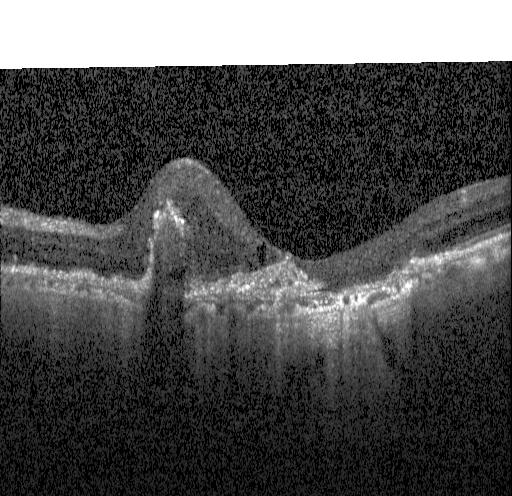 Optical coherence tomography scan. Instrument: Heidelberg Spectralis. Fovea-centered. Choroidal neovascularization (CNV).